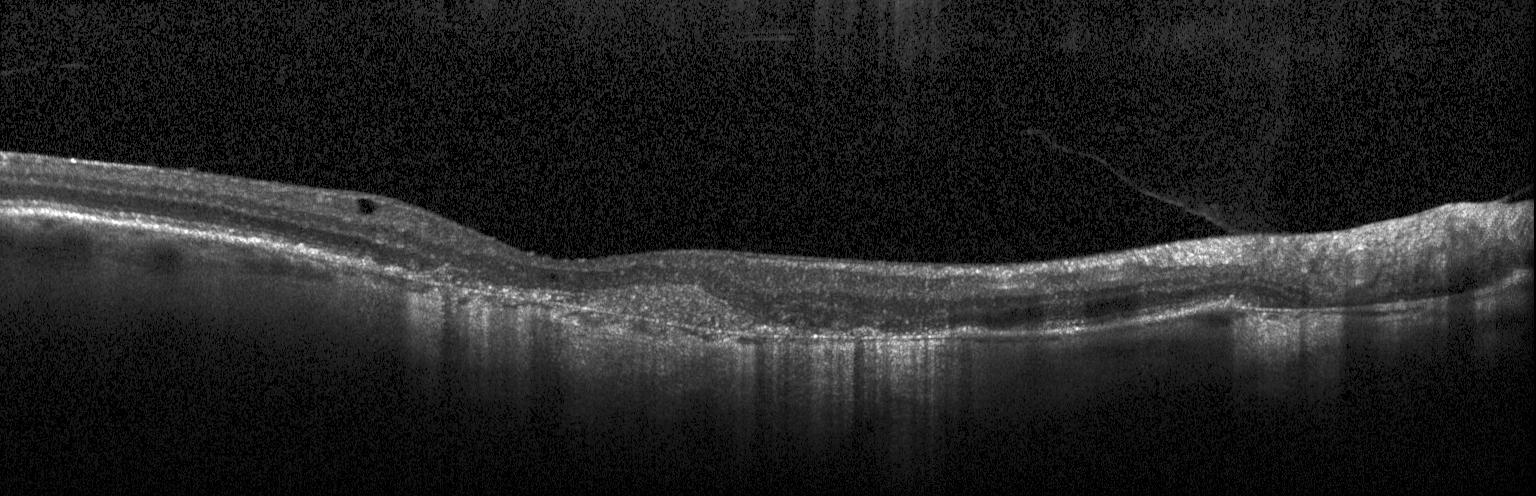

Centered on the fovea · optical coherence tomography B-scan. Assessment: a choroidal neovascular membrane.